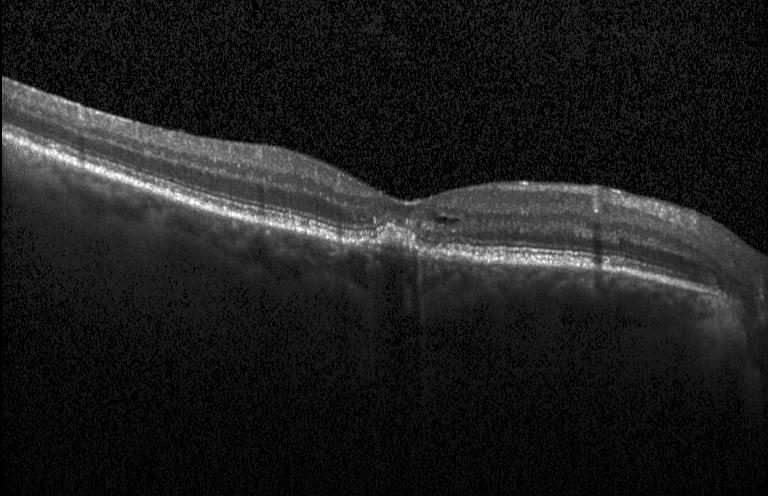
Impression: choroidal neovascularization (CNV).